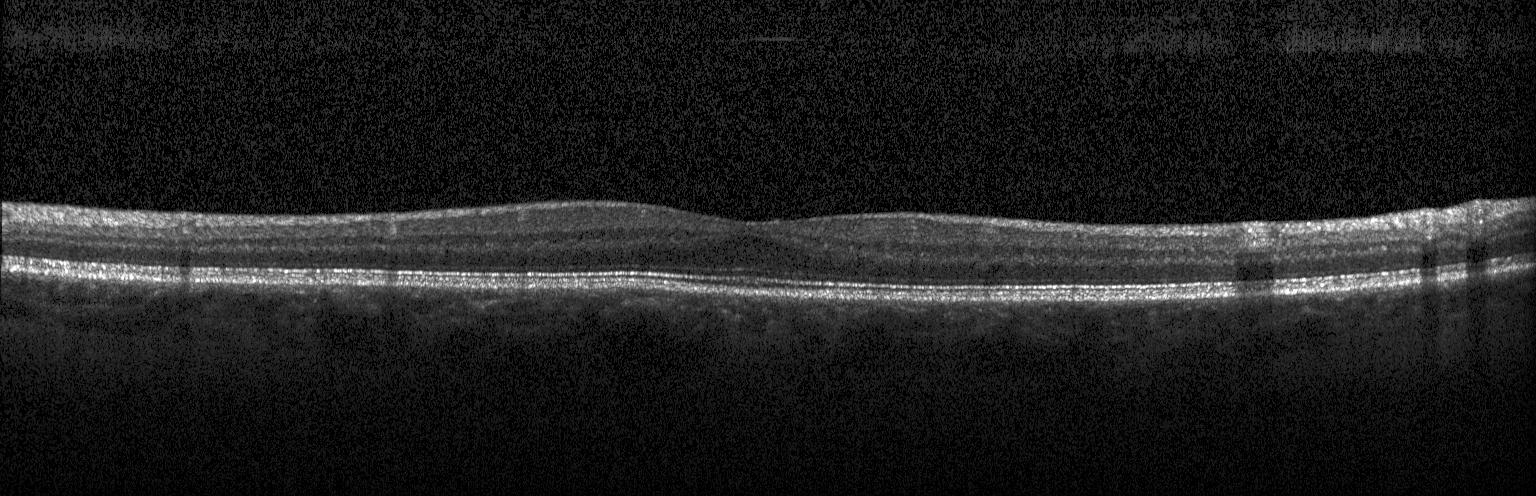

Through the macula · optical coherence tomography B-scan · acquired on a Heidelberg Spectralis — Neither choroidal neovascularization, diabetic macular edema, nor drusen.